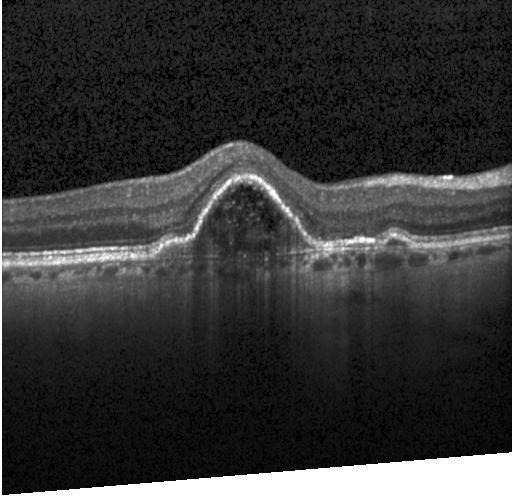
Dx: a choroidal neovascular membrane.